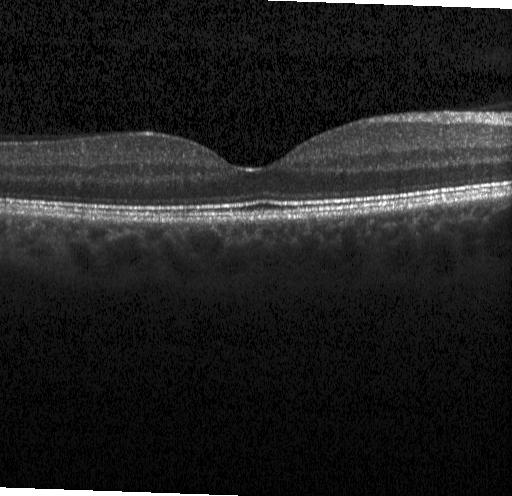 This B-scan demonstrates neither choroidal neovascularization, diabetic macular edema, nor drusen.